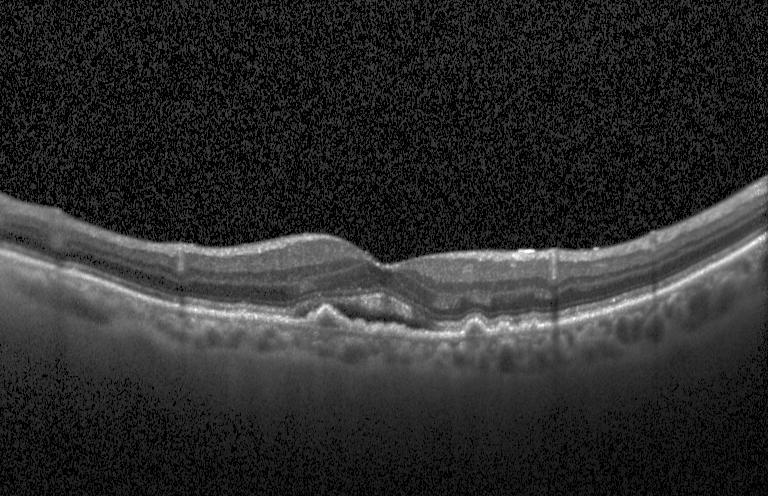 Retinal OCT B-scan. Diagnosis: choroidal neovascularization (CNV).